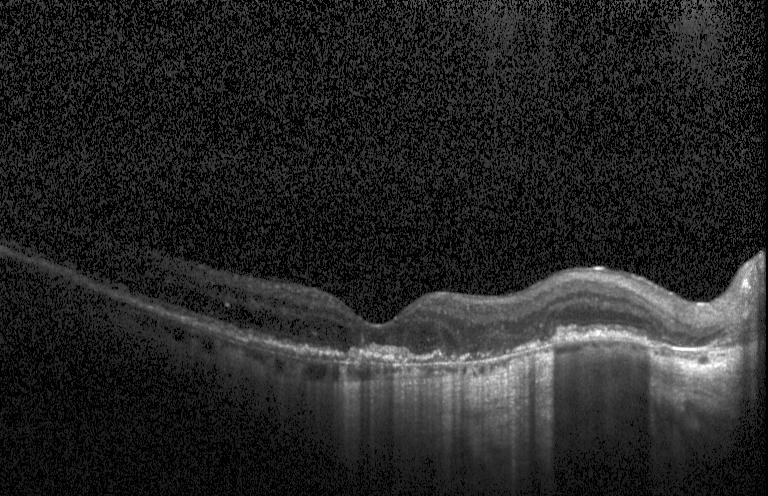
Spectral-domain optical coherence tomography, acquired on a Heidelberg Spectralis, horizontal scan through the fovea, optical coherence tomography B-scan. Finding: a choroidal neovascular membrane.